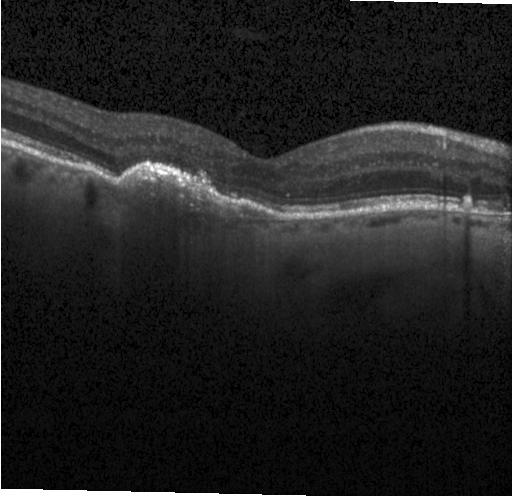

The scan shows a choroidal neovascular membrane.